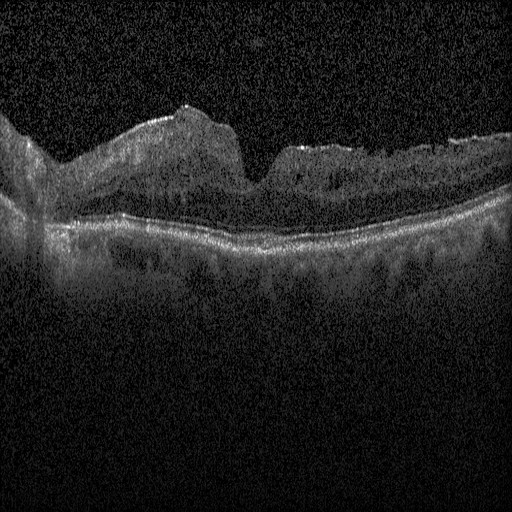

Optical coherence tomography scan.
Diagnosis: diabetic macular edema.